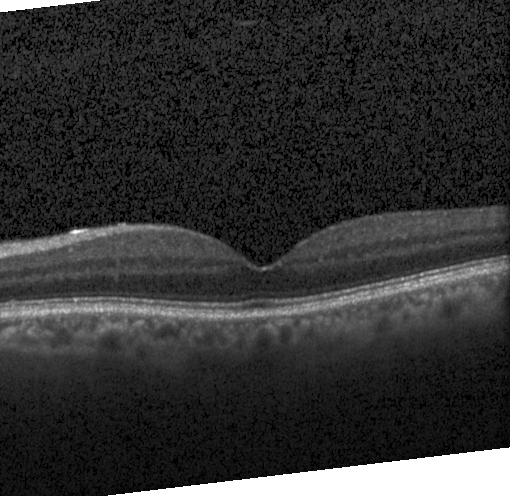
Finding: no evidence of choroidal neovascularization, diabetic macular edema, or drusen.